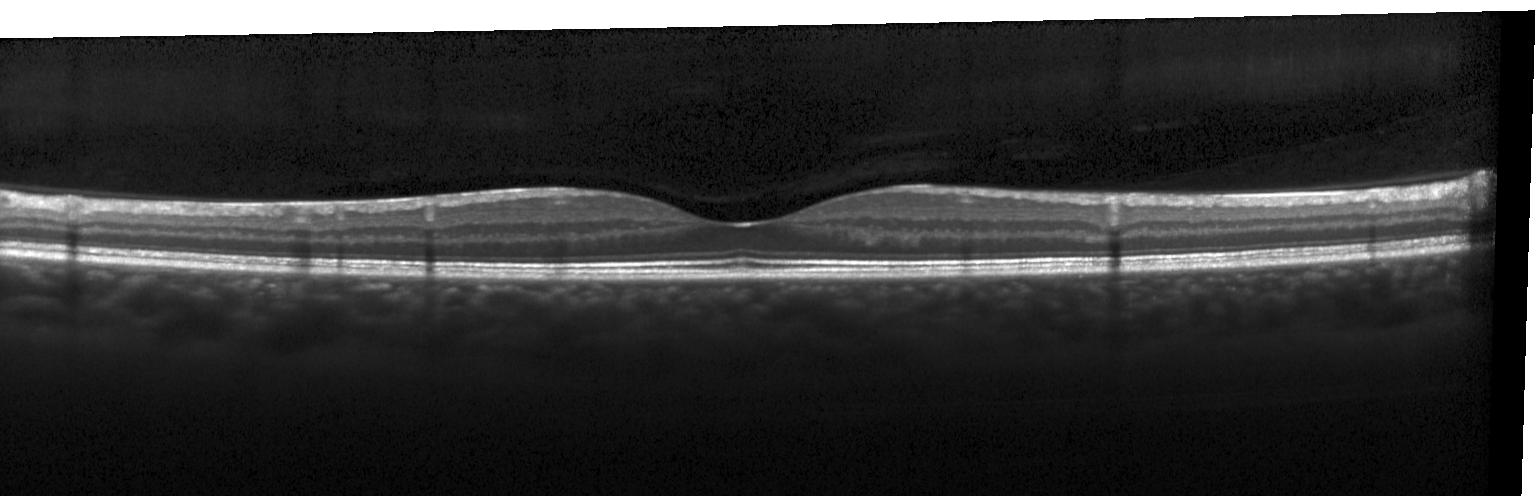

Retinal OCT B-scan.
OCT finding: no evidence of CNV, DME, or drusen.